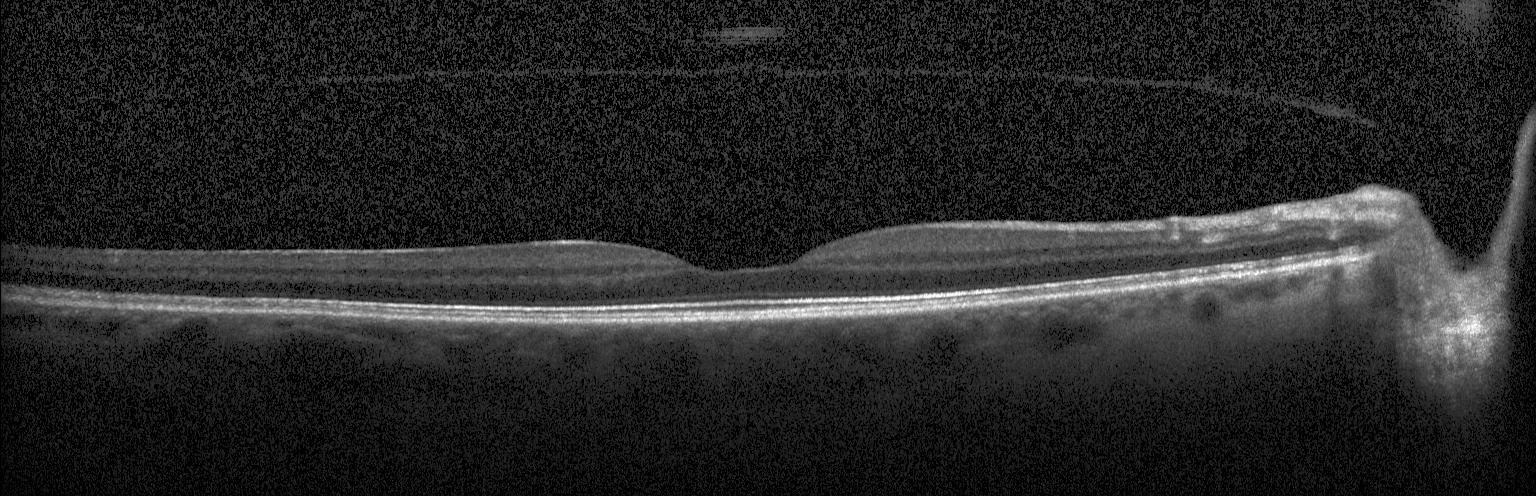
Centered on the fovea, OCT line scan — Impression: no choroidal neovascularization, diabetic macular edema, or drusen.